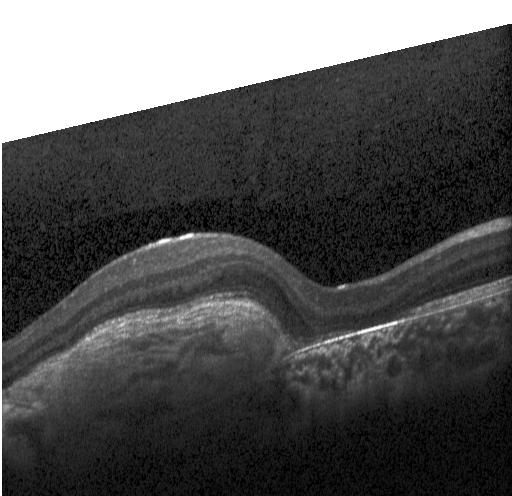 Impression: choroidal neovascularization.